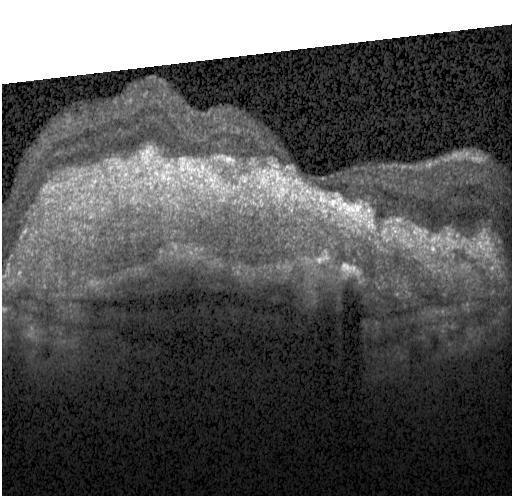
OCT scan showing choroidal neovascularization.